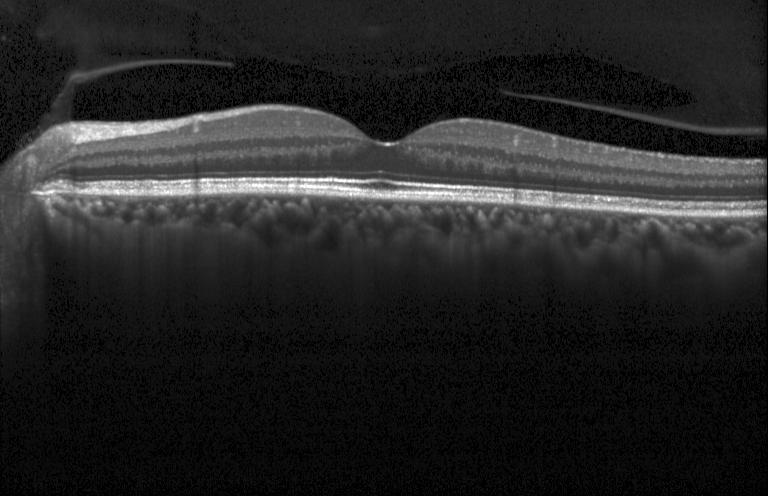
SD-OCT; OCT B-scan
No evidence of choroidal neovascularization, diabetic macular edema, or drusen.